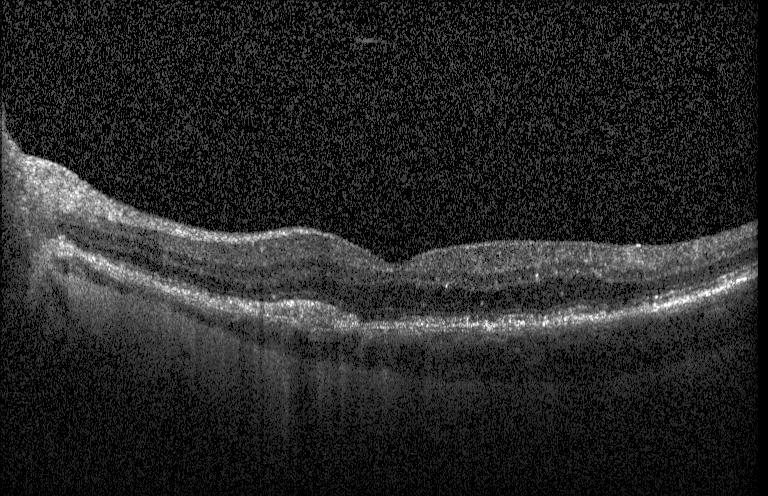 Spectral-domain optical coherence tomography. Retinal OCT B-scan. Through the macula.
Impression: a choroidal neovascular membrane.